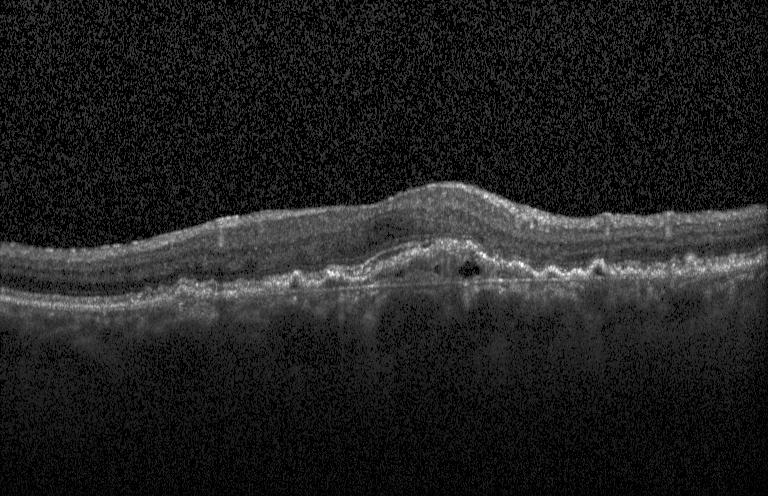 Diagnosis: a choroidal neovascular membrane.